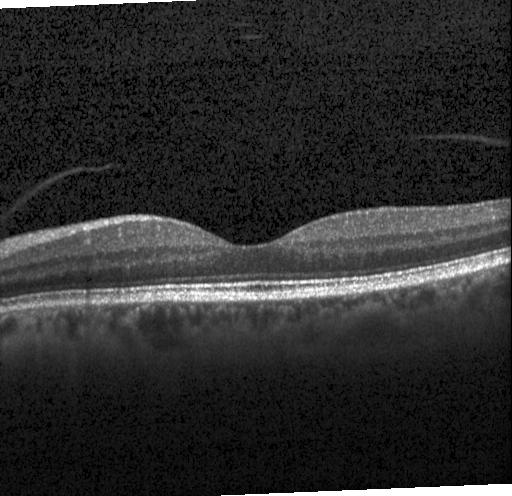

Optical coherence tomography scan · Heidelberg Spectralis · spectral-domain optical coherence tomography
Impression: neither CNV, DME, nor drusen.